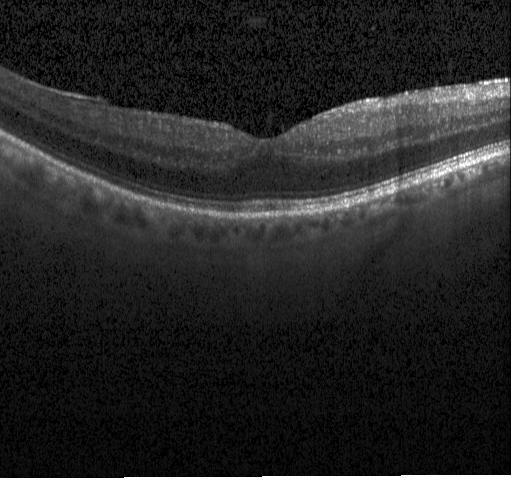

Retinal OCT cross-section showing no evidence of choroidal neovascularization, diabetic macular edema, or drusen.